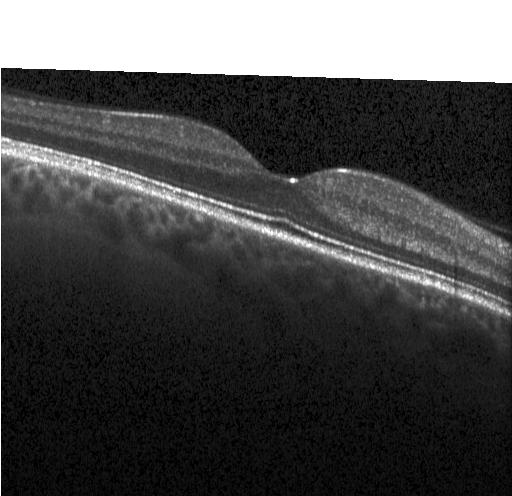

Spectral-domain OCT B-scan: no CNV, no DME, and no drusen.